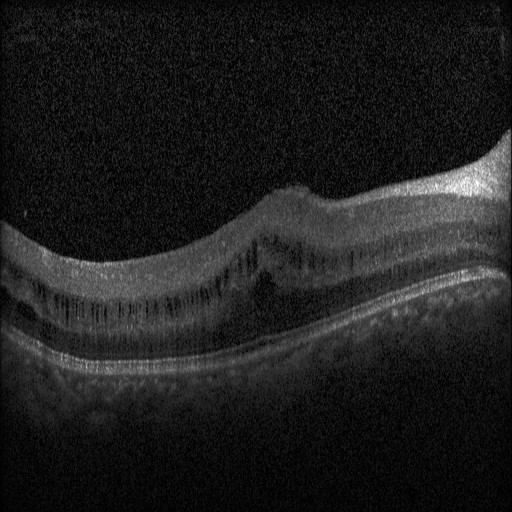

Retinal OCT B-scan · instrument: Heidelberg Spectralis. This B-scan demonstrates diabetic macular edema.